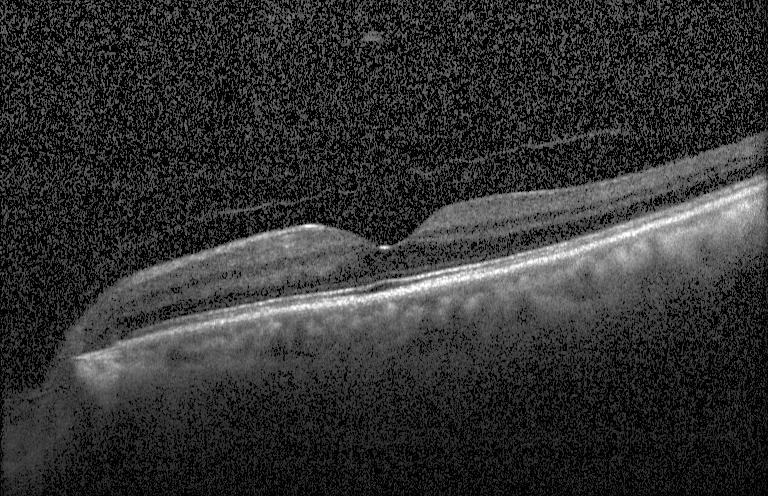
Heidelberg Spectralis; OCT line scan; fovea-centered; spectral-domain optical coherence tomography
Diagnosis: no CNV, DME, or drusen.